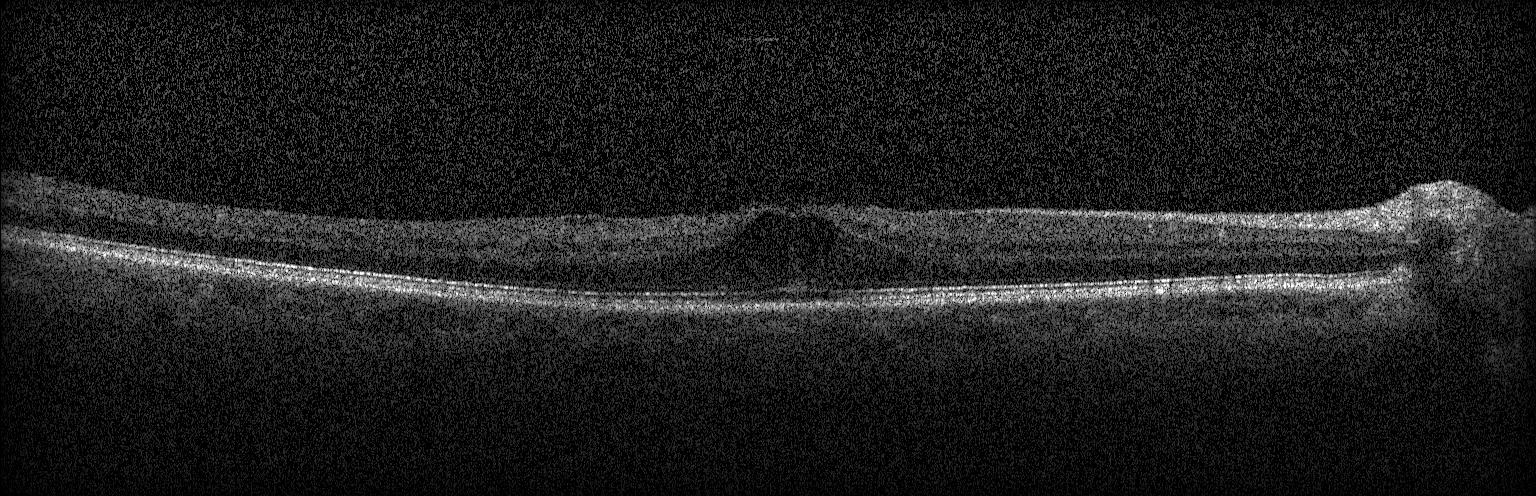
The scan shows diabetic macular edema (DME).